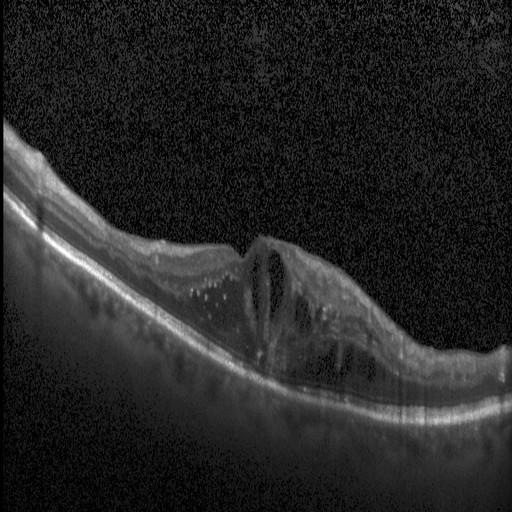
Instrument: Heidelberg Spectralis; optical coherence tomography B-scan; SD-OCT; through the macula. Diagnosis: diabetic macular edema (DME).